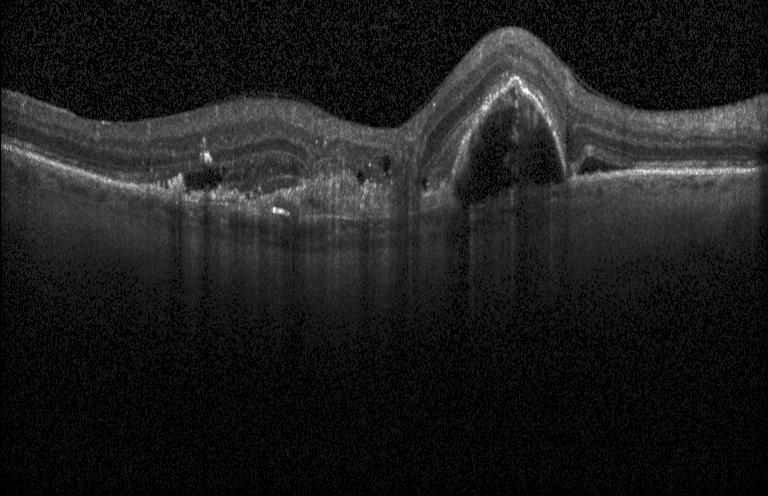

Impression: a choroidal neovascular membrane.